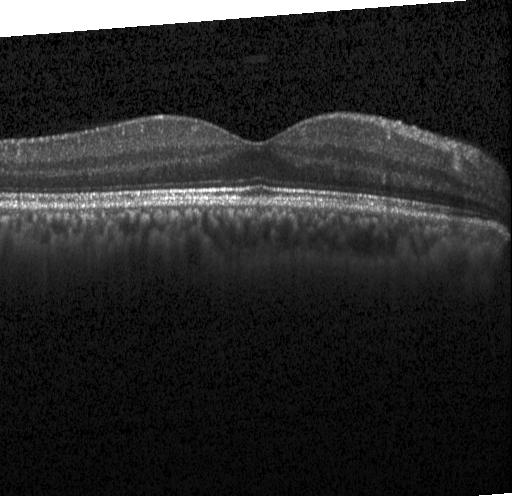
Heidelberg Spectralis, OCT line scan, spectral-domain OCT — Dx: no evidence of choroidal neovascularization, diabetic macular edema, or drusen.